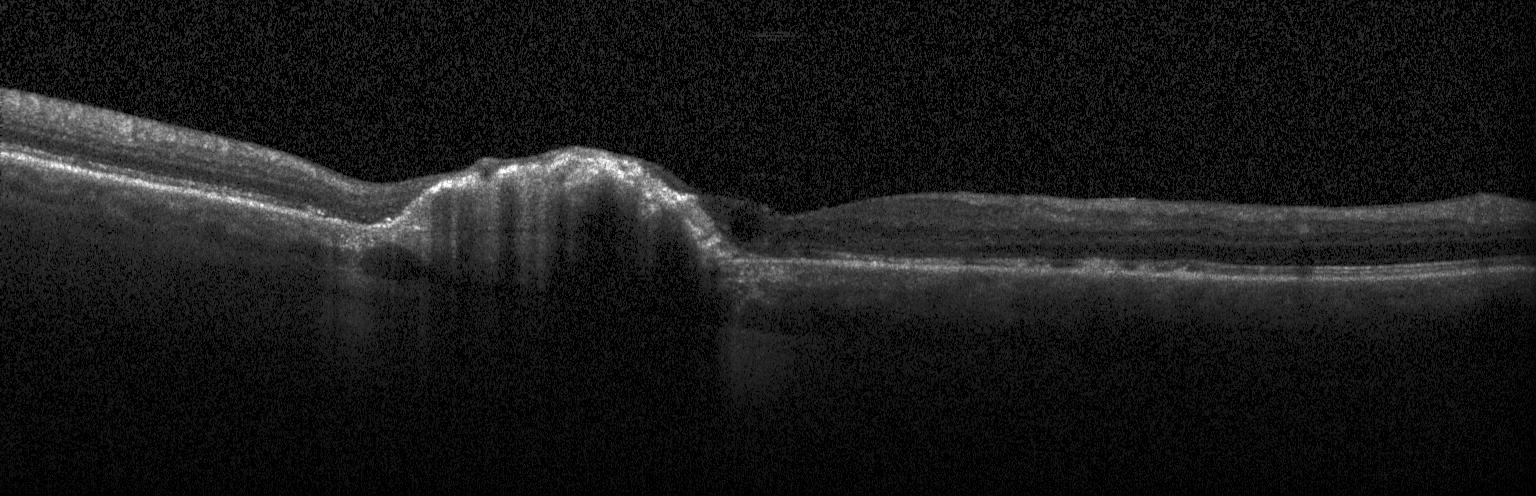
Diagnosis: a choroidal neovascular membrane.